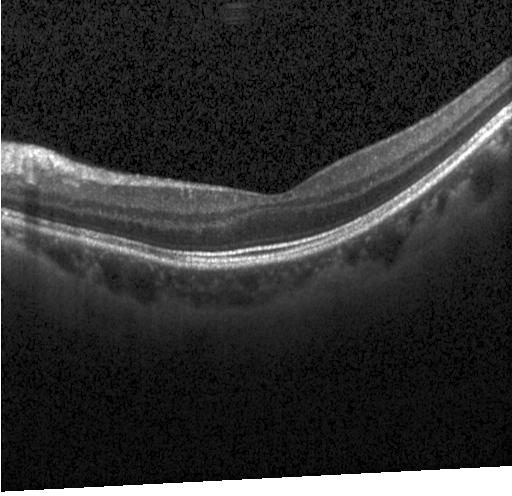

OCT line scan; macular scan — Assessment: no CNV, DME, or drusen.